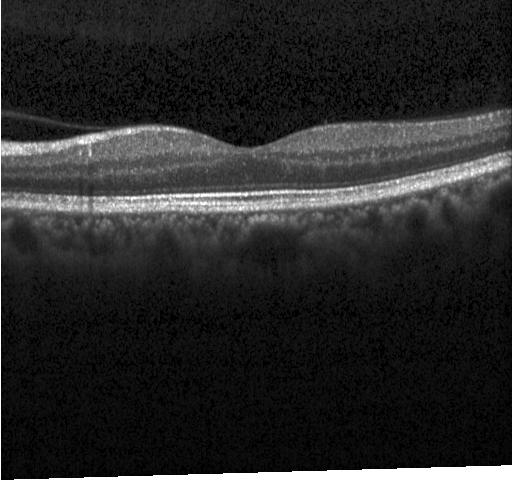
Heidelberg Spectralis · OCT line scan · spectral-domain optical coherence tomography · macular scan.
Diagnosis: no choroidal neovascularization, diabetic macular edema, or drusen.